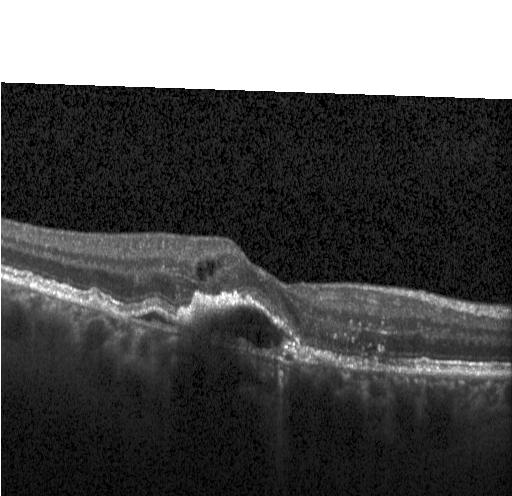

Optical coherence tomography B-scan
Diagnosis: a choroidal neovascular membrane.